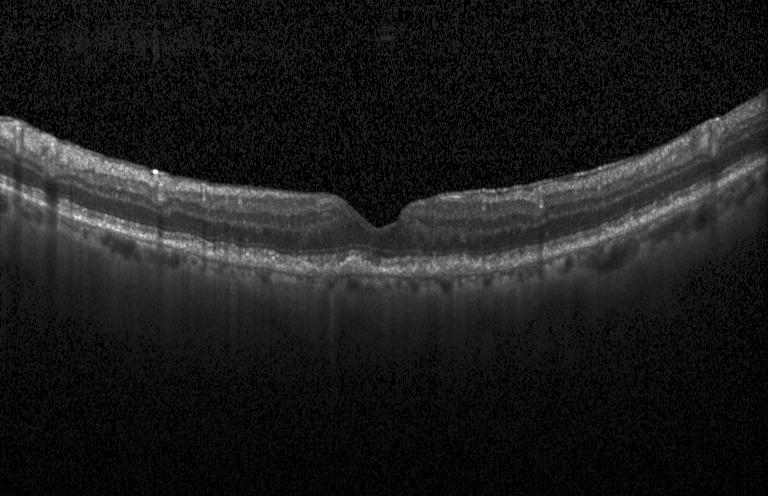 Optical coherence tomography B-scan, Heidelberg Spectralis OCT system.
Diagnosis: multiple drusen.